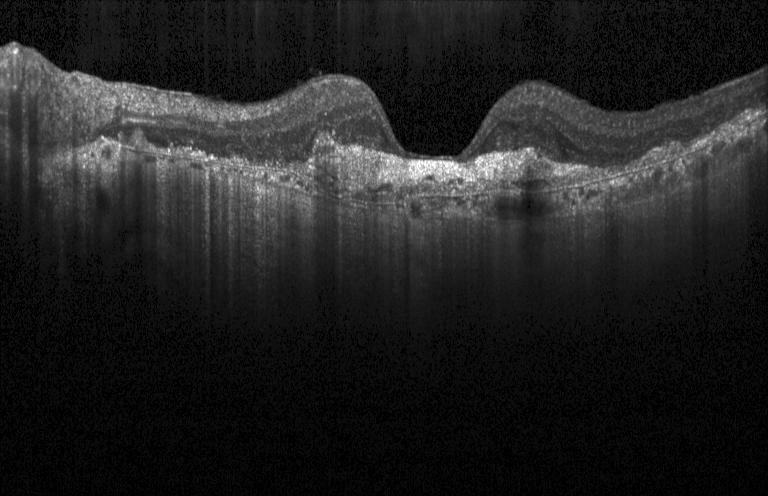

Optical coherence tomography B-scan. Horizontal scan through the fovea — Macular OCT: a choroidal neovascular membrane.